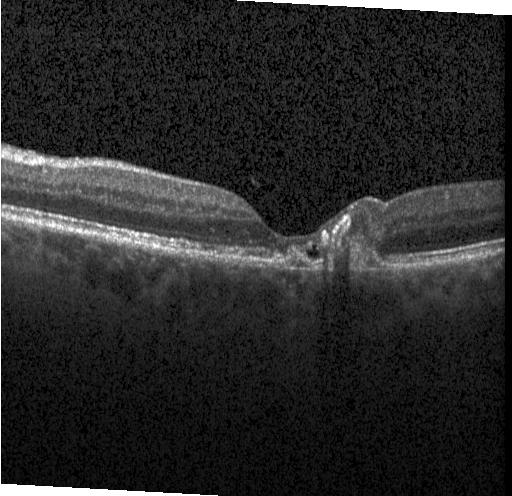 Spectral-domain OCT · through the macula · acquired on a Heidelberg Spectralis · OCT B-scan
The scan shows a choroidal neovascular membrane.